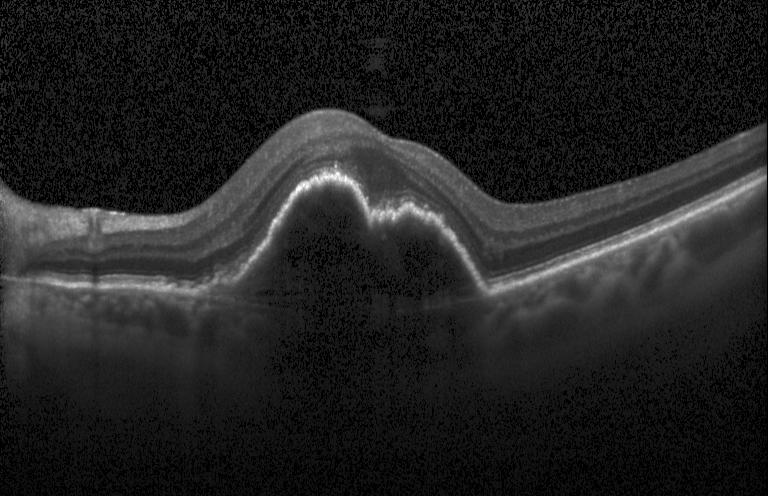

Retinal OCT cross-section; fovea-centered; SD-OCT — Assessment: a choroidal neovascular membrane.